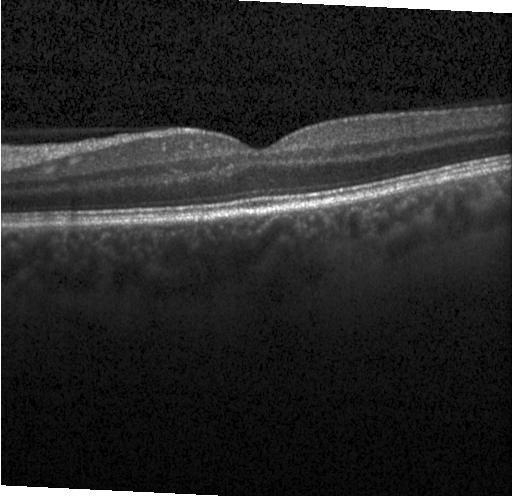

Spectral-domain optical coherence tomography. OCT line scan. Through the macula — Assessment: no CNV, no DME, and no drusen.